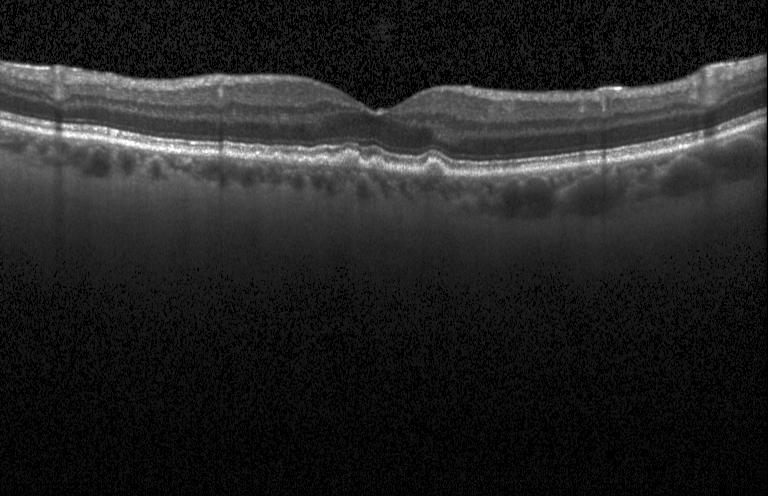 OCT B-scan. Spectral-domain optical coherence tomography. Finding: multiple drusen.